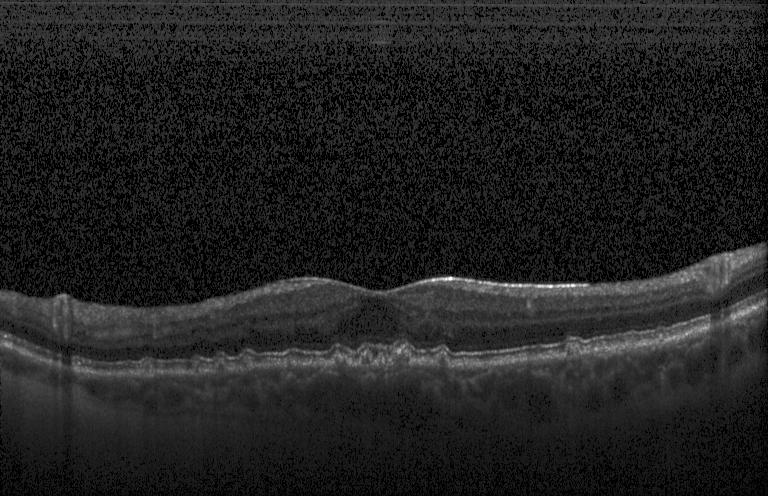

Assessment: sub-RPE drusenoid deposits.